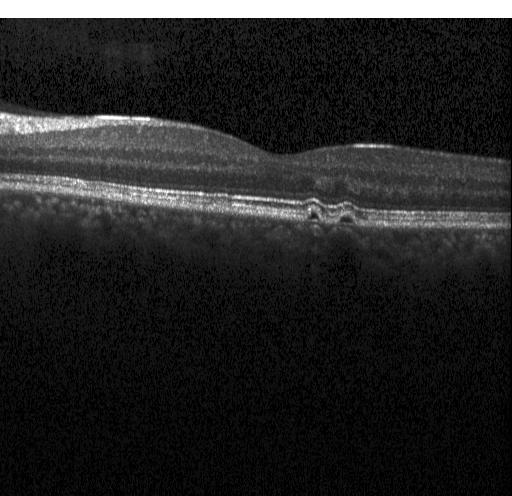

The scan shows multiple drusen.